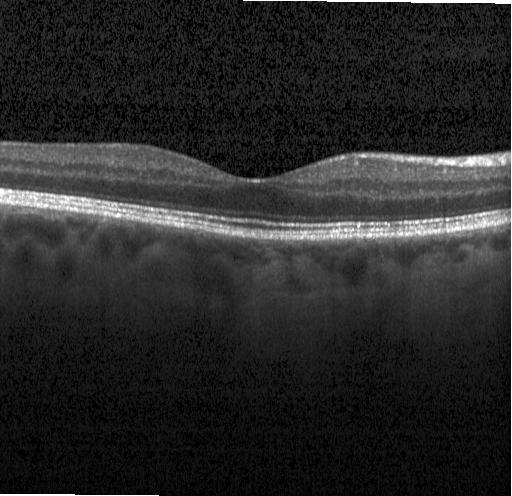 Spectral-domain OCT. Macular scan. OCT line scan. Heidelberg Spectralis OCT system
Assessment: no choroidal neovascularization, no diabetic macular edema, and no drusen.